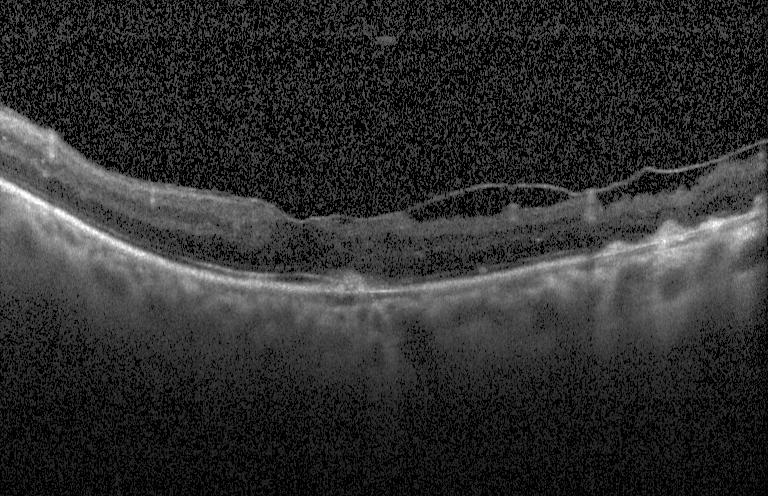

OCT line scan
Assessment: choroidal neovascularization (CNV).